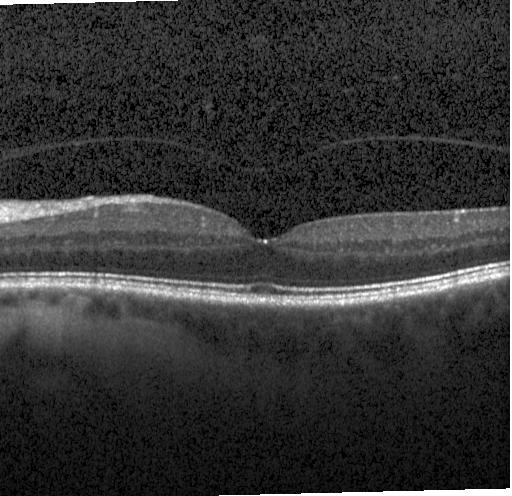 Spectral-domain OCT B-scan: neither choroidal neovascularization, diabetic macular edema, nor drusen.